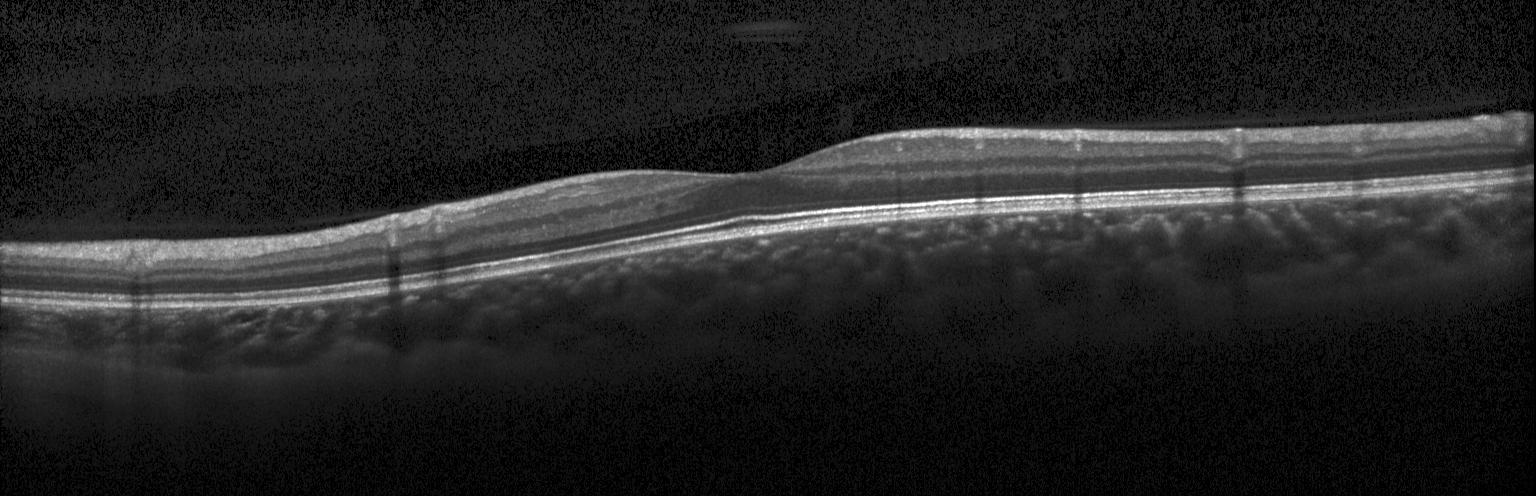

Optical coherence tomography B-scan. Instrument: Heidelberg Spectralis — The scan shows no CNV, DME, or drusen.